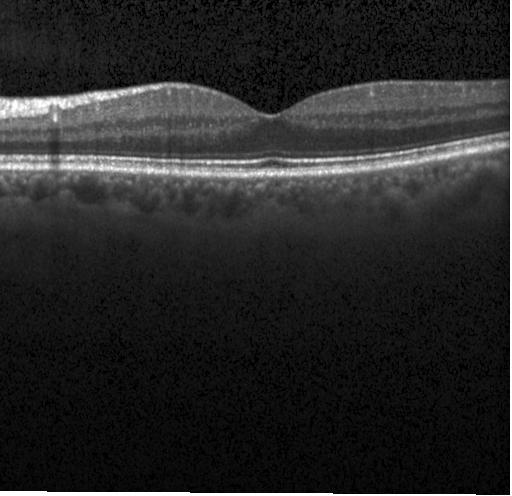
Spectral-domain optical coherence tomography · OCT B-scan. No evidence of choroidal neovascularization, diabetic macular edema, or drusen.